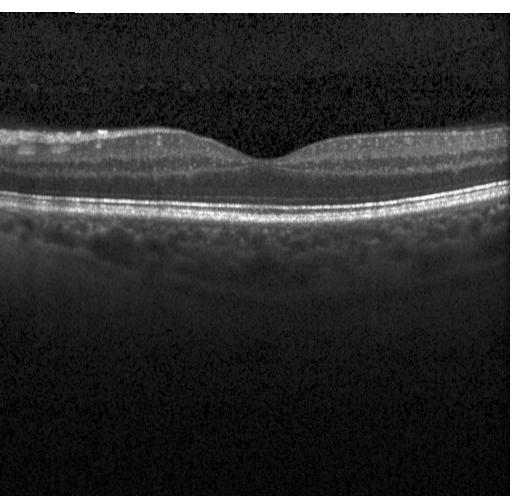

Macular scan; OCT B-scan; acquired on a Heidelberg Spectralis; SD-OCT — Impression: no choroidal neovascularization, no diabetic macular edema, and no drusen.